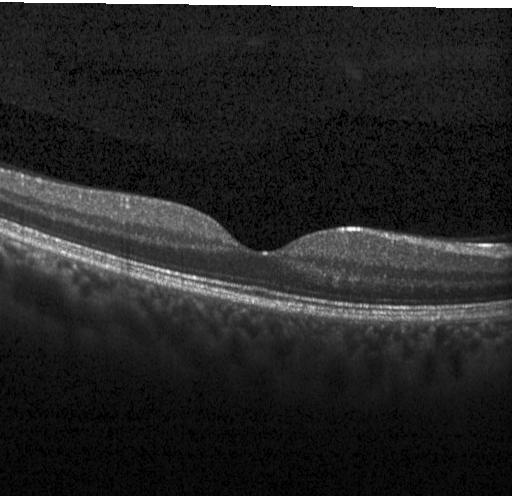 Retinal OCT cross-section. Assessment: no choroidal neovascularization, diabetic macular edema, or drusen.